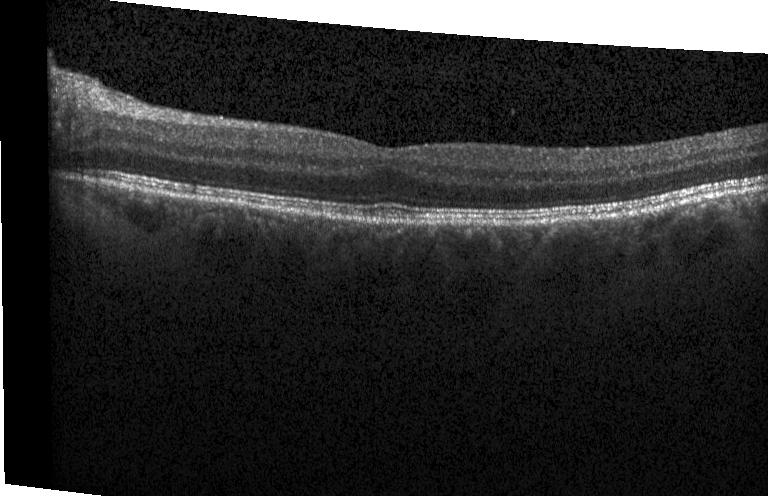 Fovea-centered; retinal OCT cross-section; acquired on a Heidelberg Spectralis — Diagnosis: no evidence of choroidal neovascularization, diabetic macular edema, or drusen.